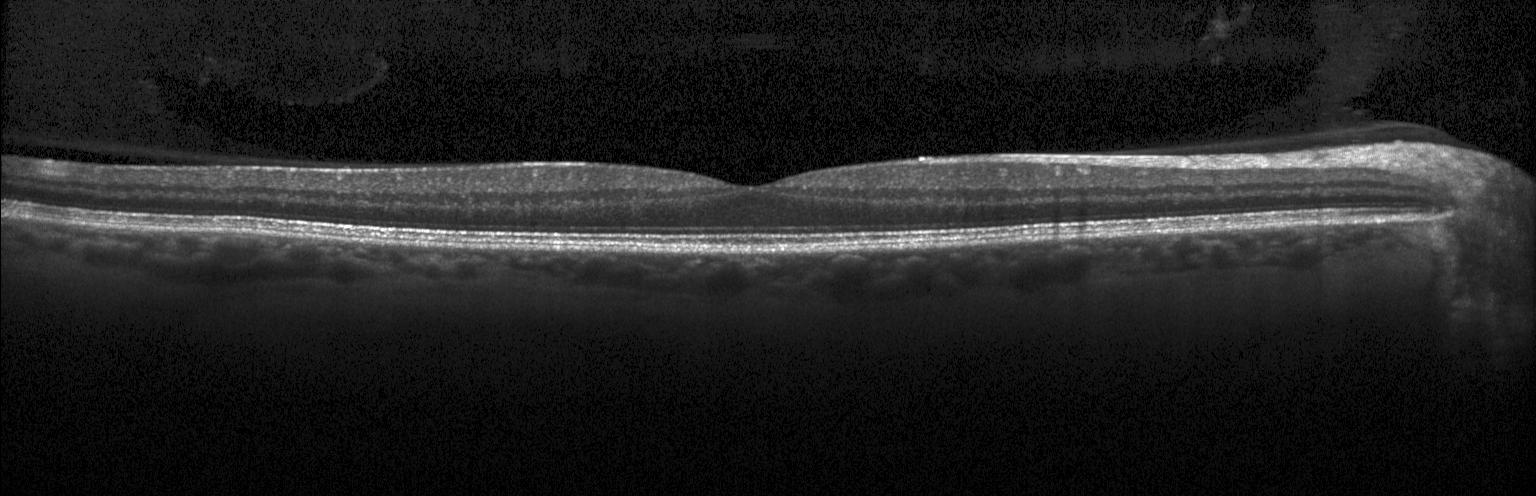

Spectral-domain OCT, centered on the fovea, OCT line scan. Impression: no evidence of choroidal neovascularization, diabetic macular edema, or drusen.